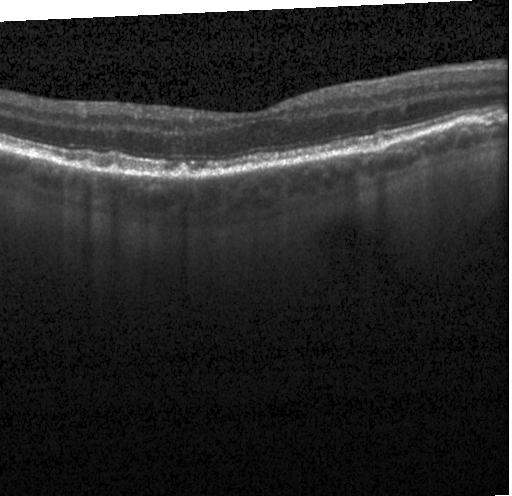
OCT B-scan; through the macula.
Drusen.